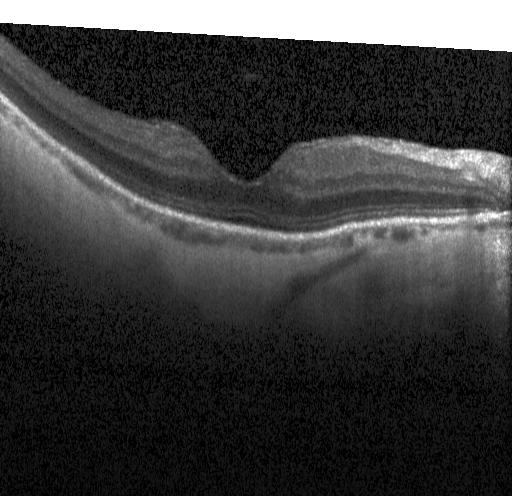 OCT line scan. Horizontal scan through the fovea
Finding: no choroidal neovascularization, no diabetic macular edema, and no drusen.